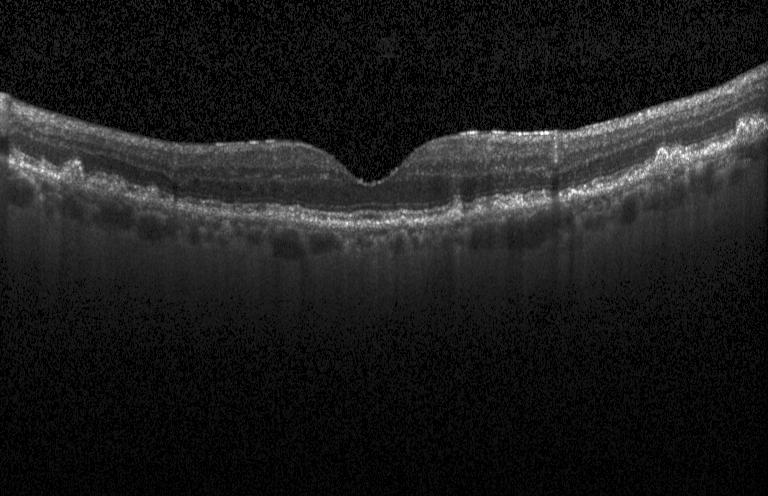 Optical coherence tomography B-scan — This B-scan demonstrates sub-RPE drusenoid deposits.